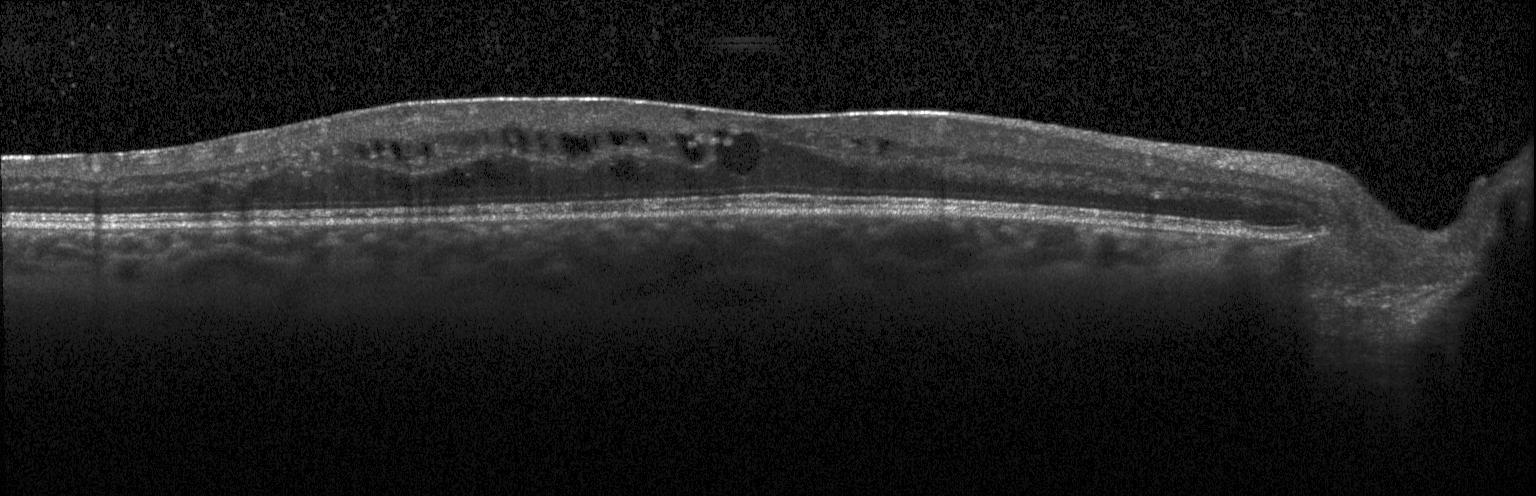 Retinal OCT cross-section
Diagnosis: diabetic macular edema.